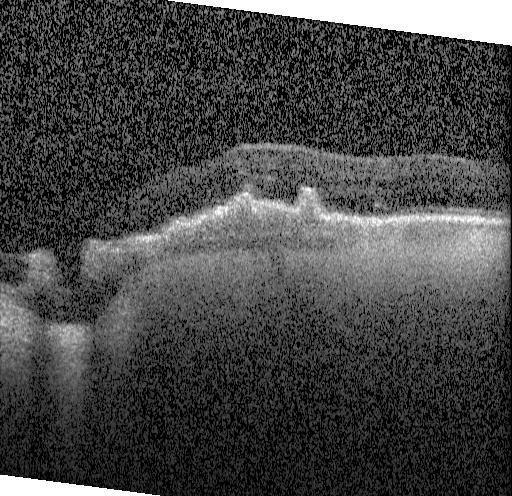
Retinal OCT cross-section.
CNV.